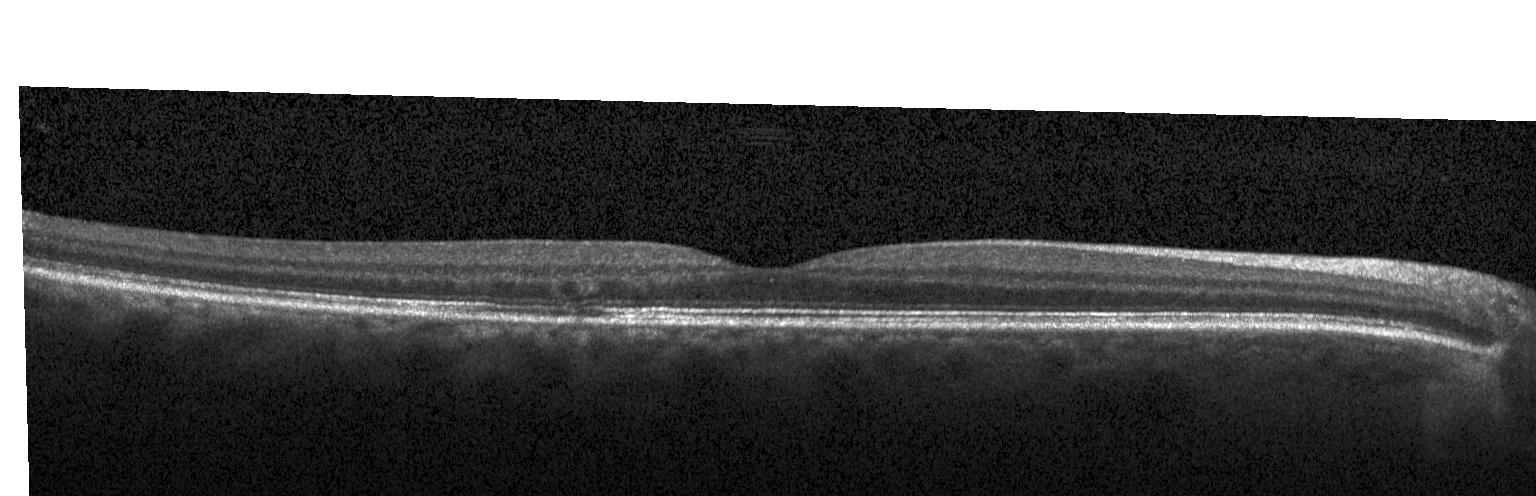
OCT B-scan; macular scan; SD-OCT; instrument: Heidelberg Spectralis. Finding: neither choroidal neovascularization, diabetic macular edema, nor drusen.